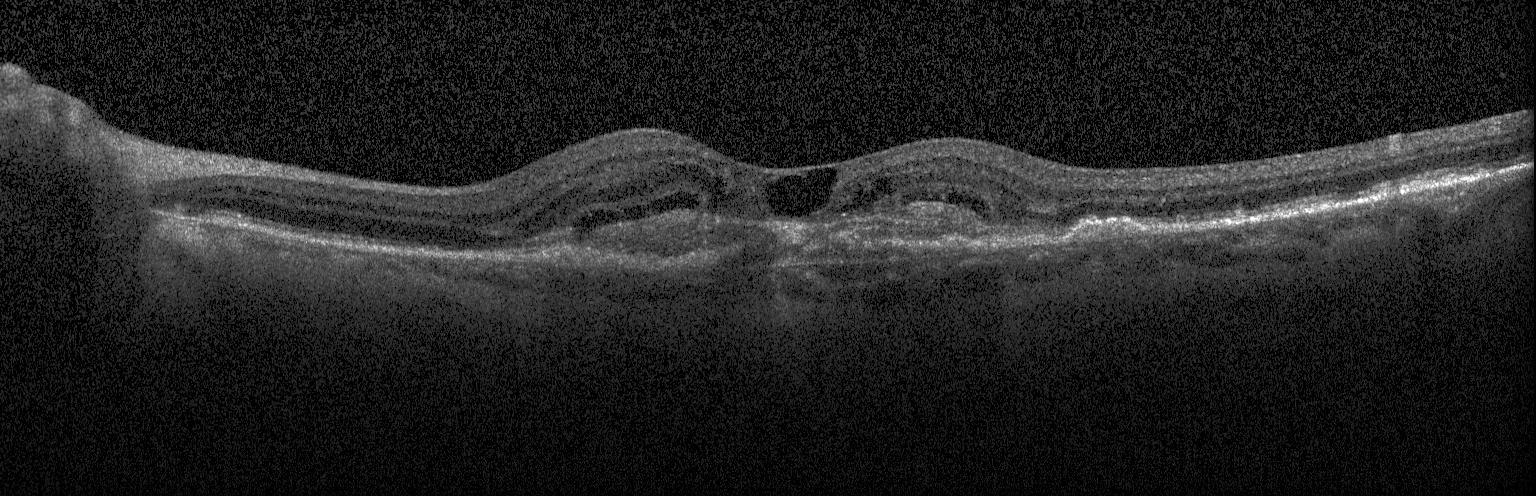
Optical coherence tomography scan. Diagnosis: choroidal neovascularization (CNV).